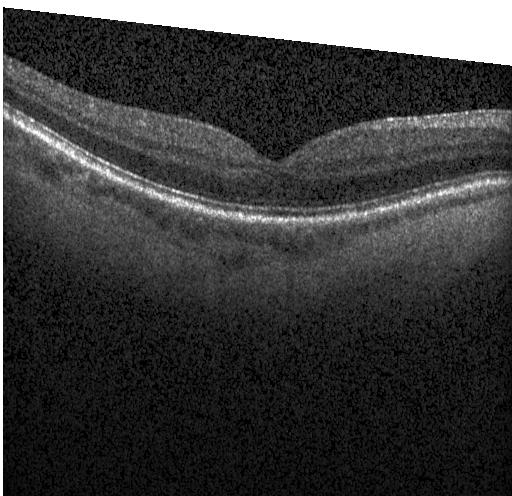

Diagnosis: no CNV, no DME, and no drusen.